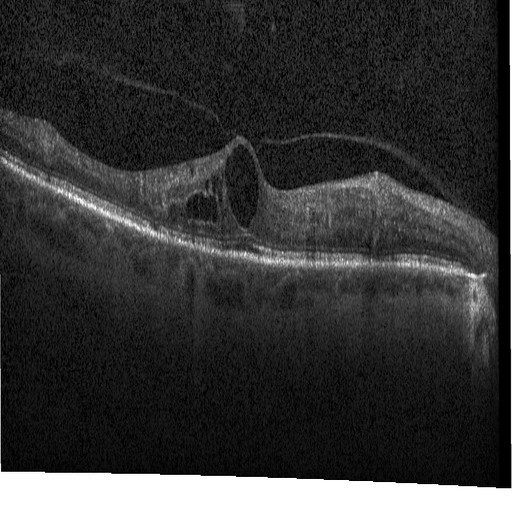
Diabetic macular edema.